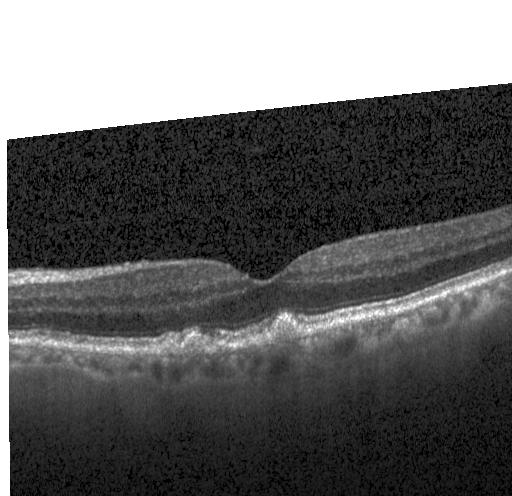
Through the macula; spectral-domain OCT; retinal OCT cross-section; Heidelberg Spectralis — Finding: multiple drusen.